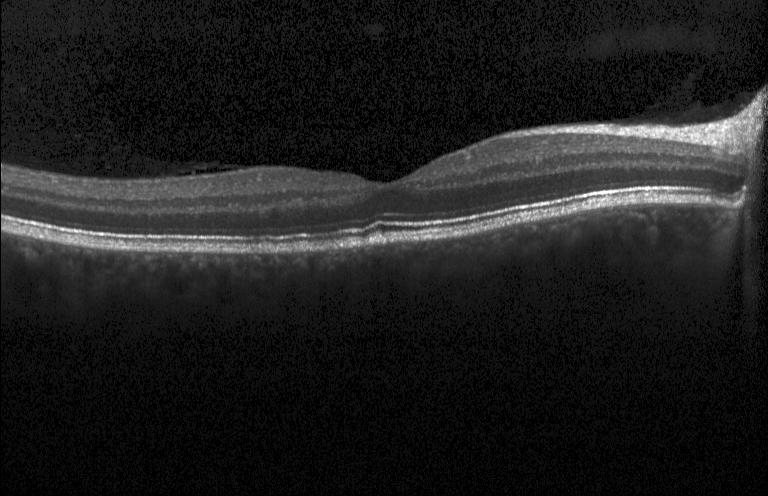

The scan shows neither choroidal neovascularization, diabetic macular edema, nor drusen.